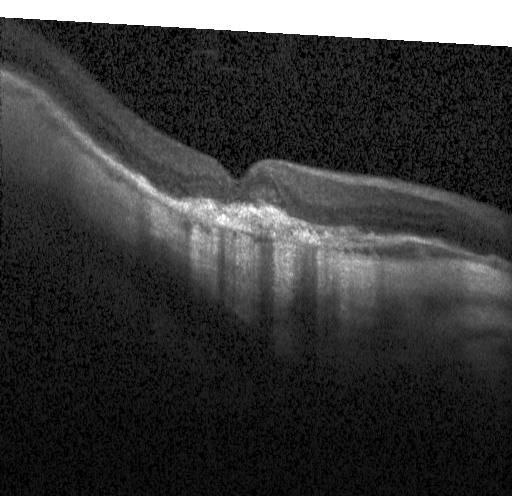

Heidelberg Spectralis; retinal OCT cross-section; spectral-domain OCT. The scan shows a choroidal neovascular membrane.